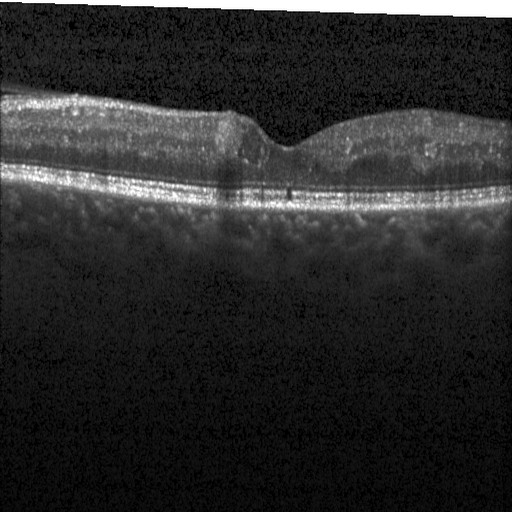
Centered on the fovea, Heidelberg Spectralis, optical coherence tomography scan — Macular OCT: diabetic macular edema (DME).